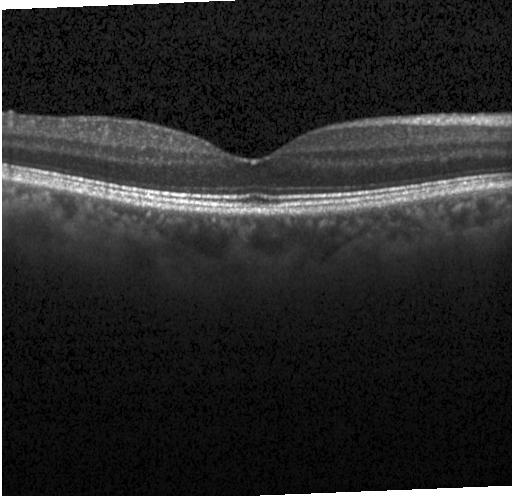 Centered on the fovea, SD-OCT, OCT line scan — Impression: no CNV, no DME, and no drusen.